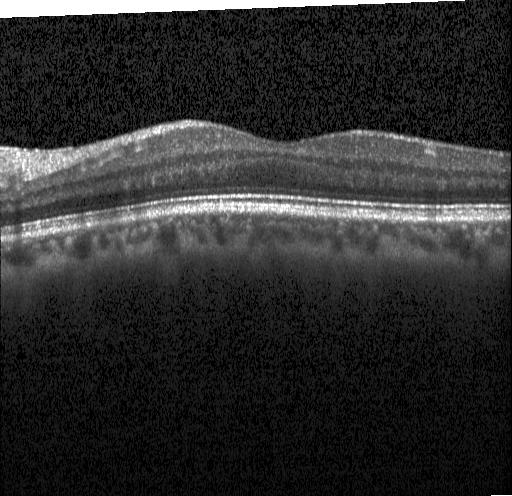 Heidelberg Spectralis OCT system, fovea-centered, optical coherence tomography scan, SD-OCT. Impression: no CNV, no DME, and no drusen.